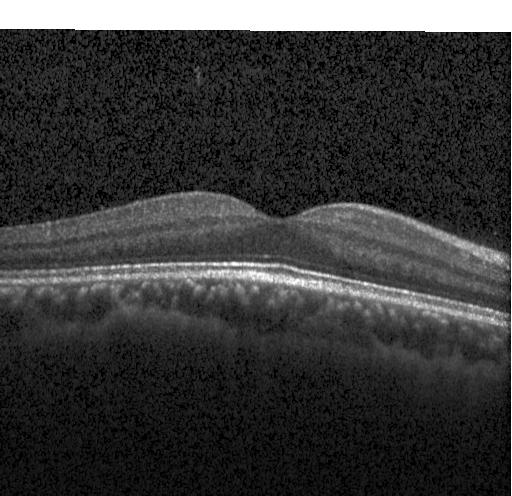
Retinal OCT cross-section. Fovea-centered. Heidelberg Spectralis. The scan shows neither choroidal neovascularization, diabetic macular edema, nor drusen.